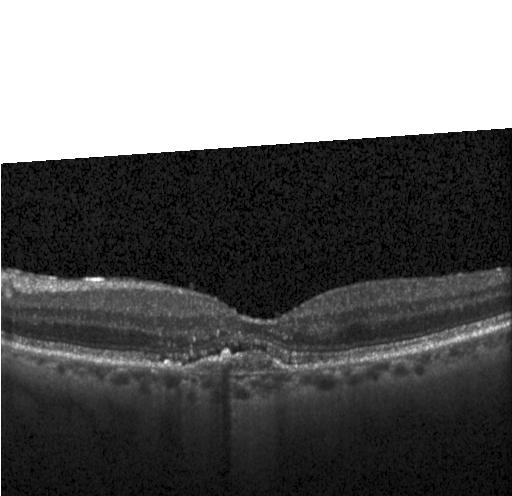

Macular OCT: a choroidal neovascular membrane.